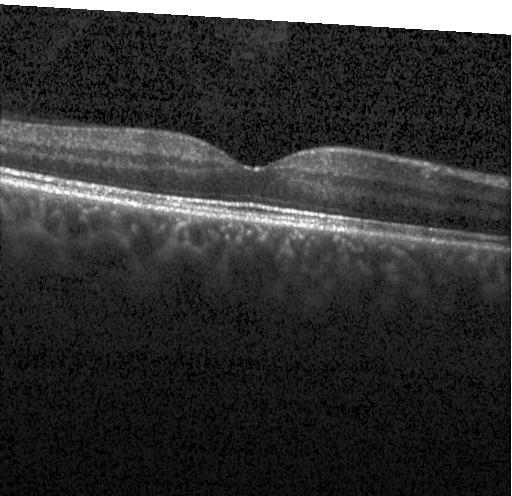

Optical coherence tomography B-scan. Diagnosis: neither CNV, DME, nor drusen.